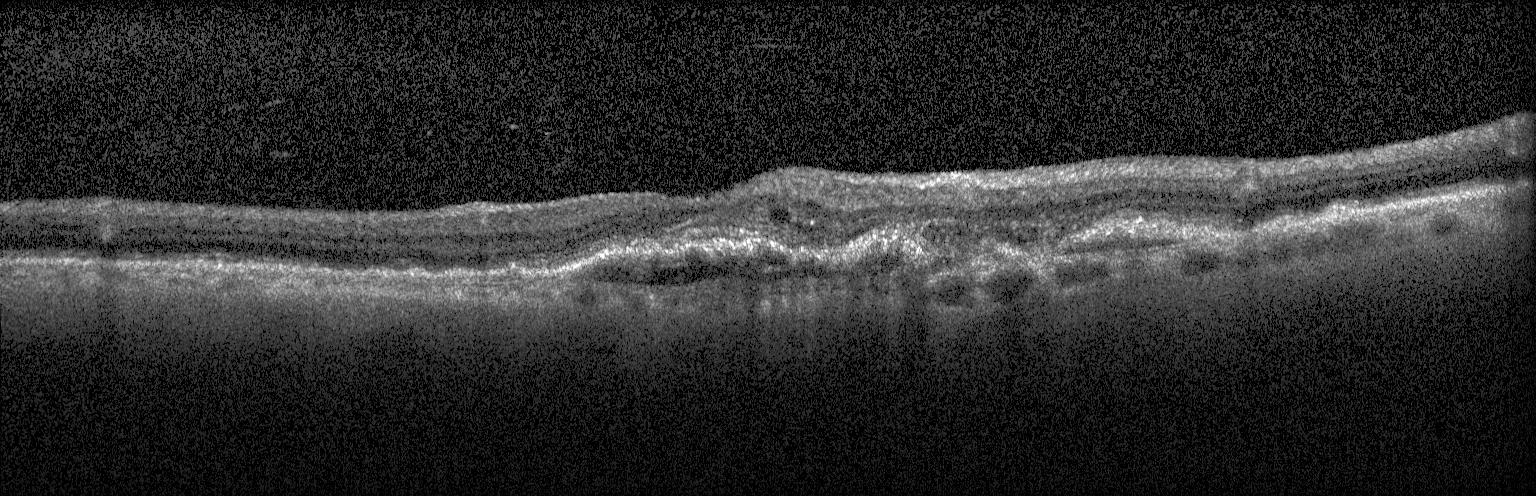

Spectral-domain optical coherence tomography · through the macula · retinal OCT B-scan · acquired on a Heidelberg Spectralis — Finding: a choroidal neovascular membrane.